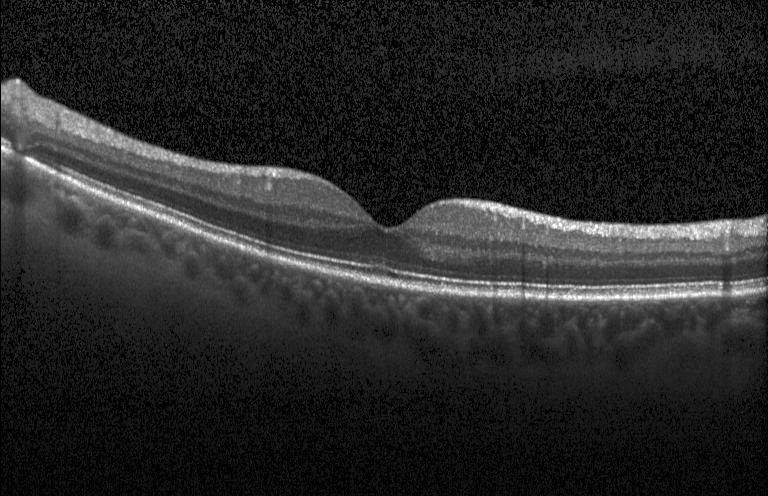 Dx: no choroidal neovascularization, no diabetic macular edema, and no drusen.